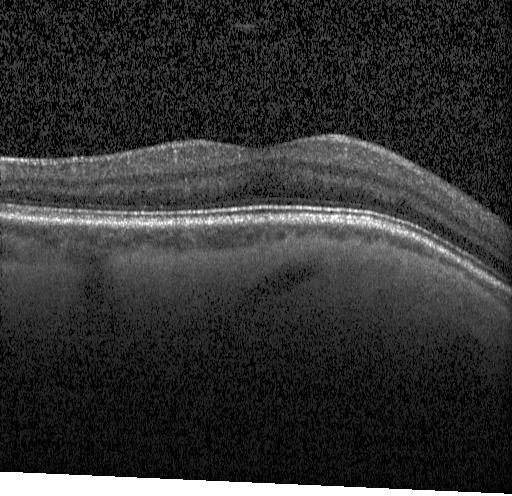

Retinal OCT cross-section. Horizontal scan through the fovea — This B-scan demonstrates no choroidal neovascularization, no diabetic macular edema, and no drusen.